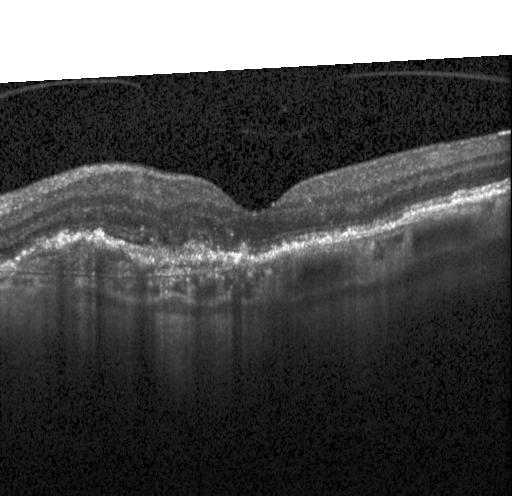
Horizontal scan through the fovea; acquired on a Heidelberg Spectralis; OCT line scan; SD-OCT. The scan shows a choroidal neovascular membrane.